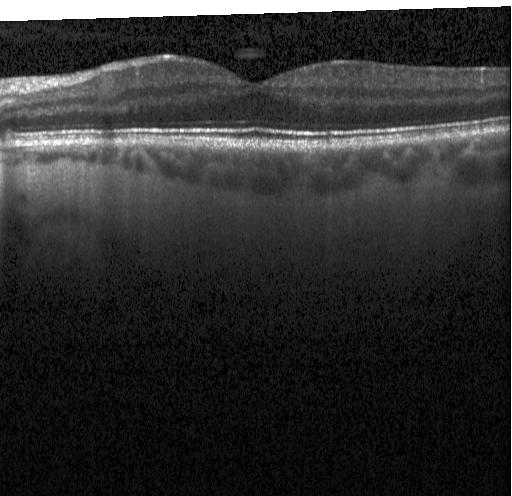 Acquired on a Heidelberg Spectralis, optical coherence tomography scan, centered on the fovea, spectral-domain OCT — Diagnosis: no CNV, no DME, and no drusen.